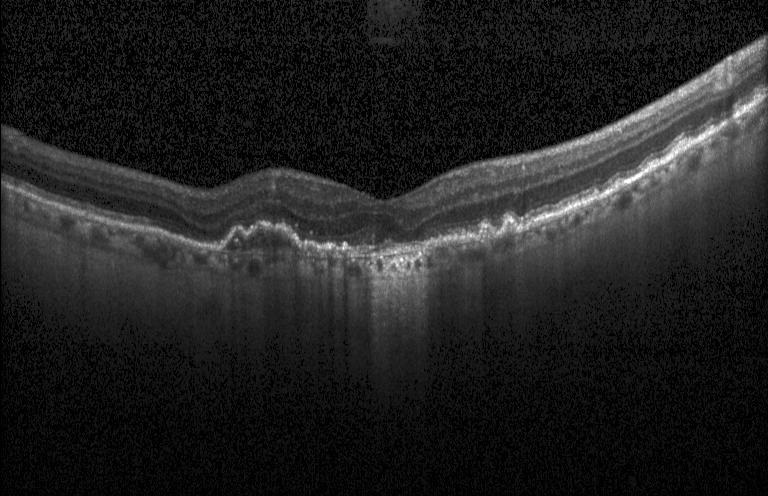
Impression: CNV.